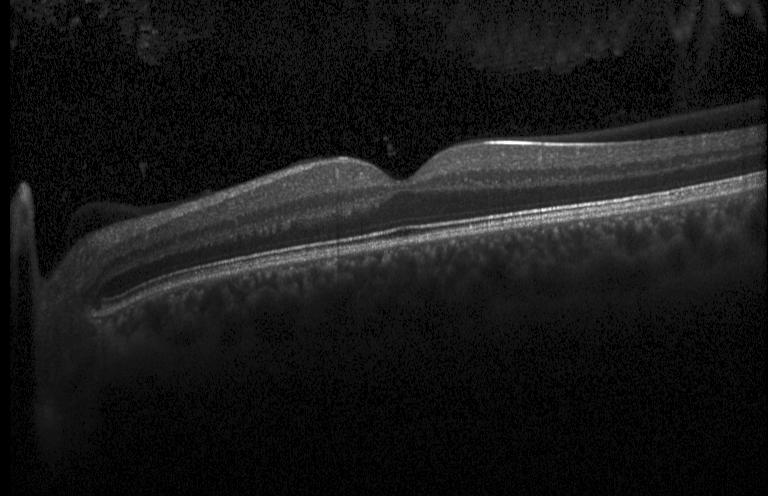
Acquired on a Heidelberg Spectralis; fovea-centered; spectral-domain optical coherence tomography; optical coherence tomography B-scan
This B-scan demonstrates no evidence of CNV, DME, or drusen.